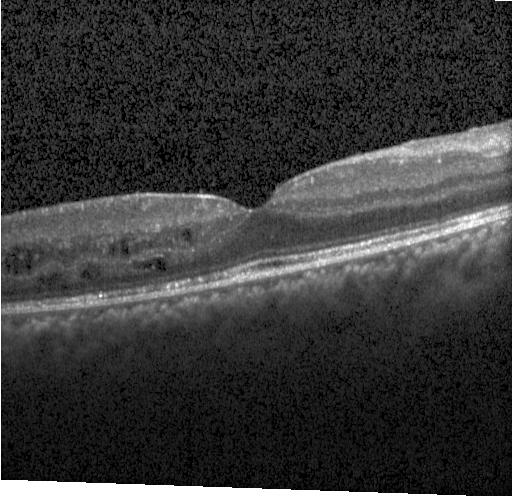 Retinal OCT B-scan; spectral-domain optical coherence tomography; instrument: Heidelberg Spectralis. Diagnosis: diabetic macular edema.